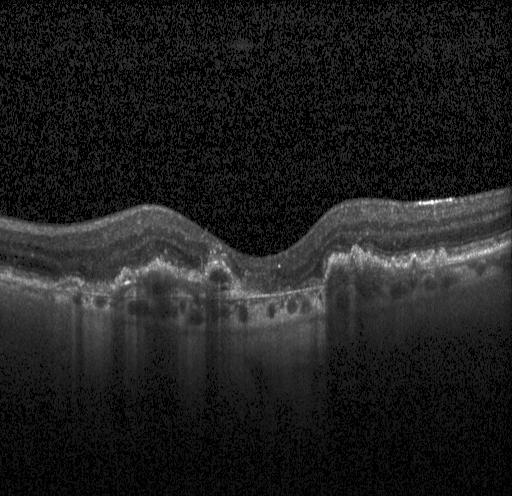
Diagnosis: a choroidal neovascular membrane.